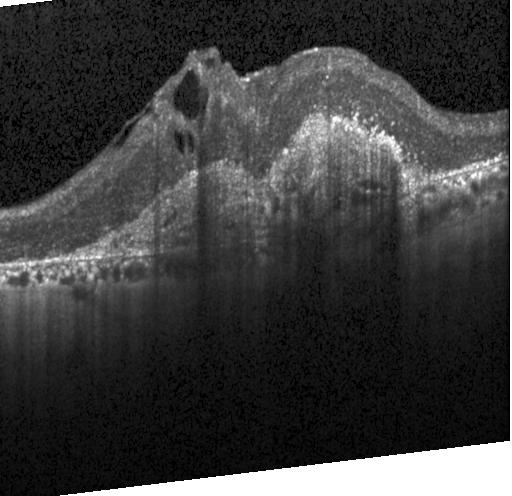

Dx: CNV.